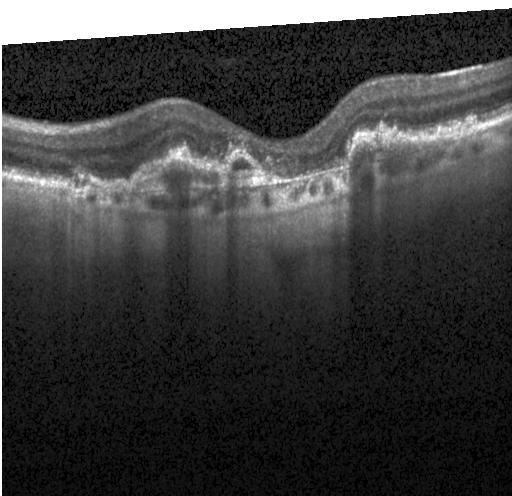
The scan shows a choroidal neovascular membrane.